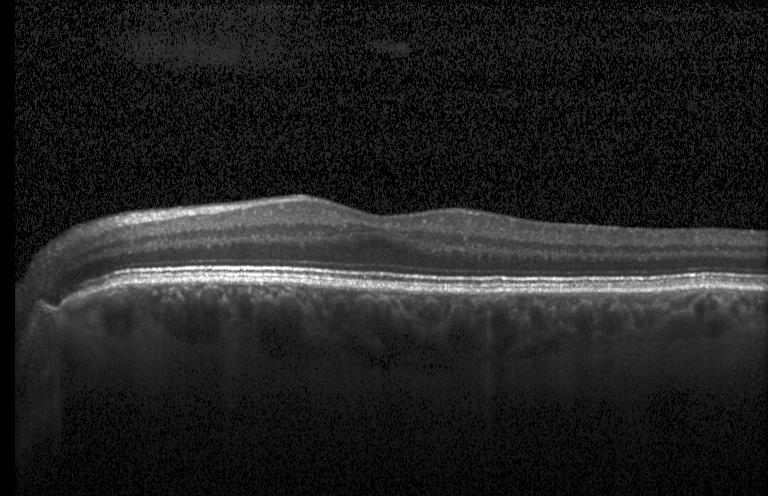
OCT B-scan, centered on the fovea, instrument: Heidelberg Spectralis. The scan shows no evidence of choroidal neovascularization, diabetic macular edema, or drusen.